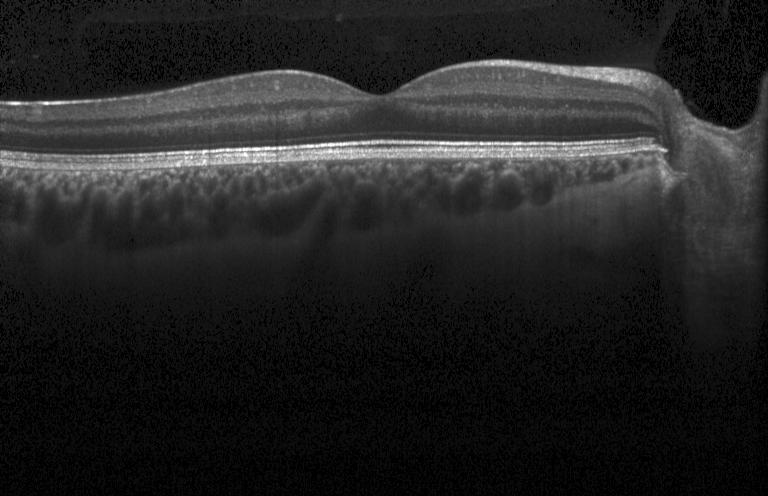
Optical coherence tomography scan; Heidelberg Spectralis OCT system
This B-scan demonstrates neither choroidal neovascularization, diabetic macular edema, nor drusen.